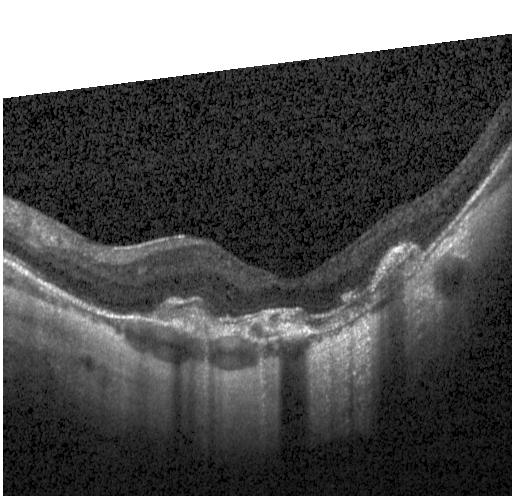
Dx: a choroidal neovascular membrane.